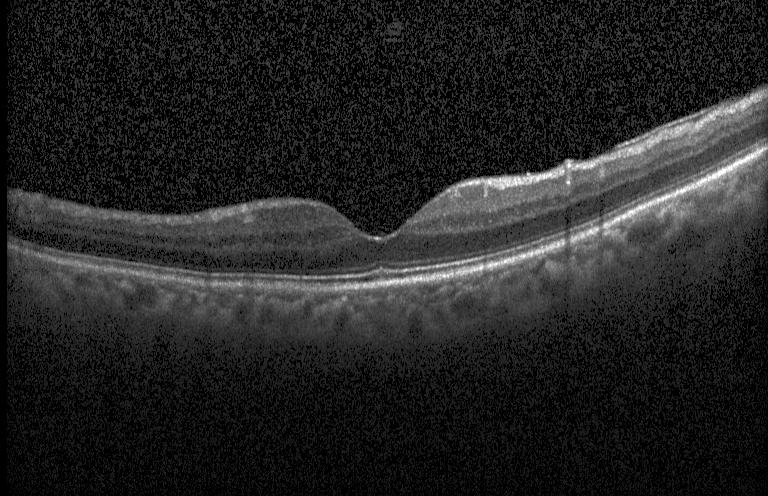

OCT line scan.
Diagnosis: neither CNV, DME, nor drusen.